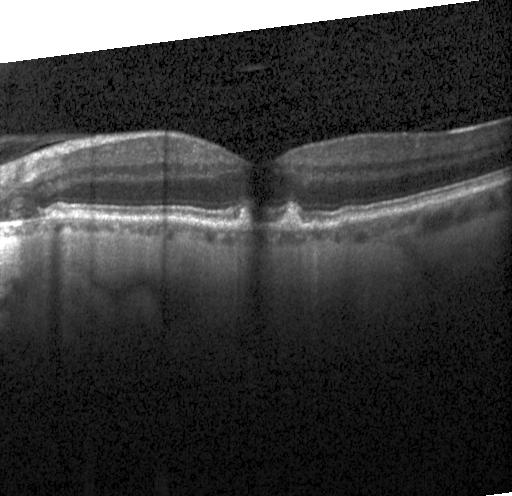

Macular OCT: multiple drusen.